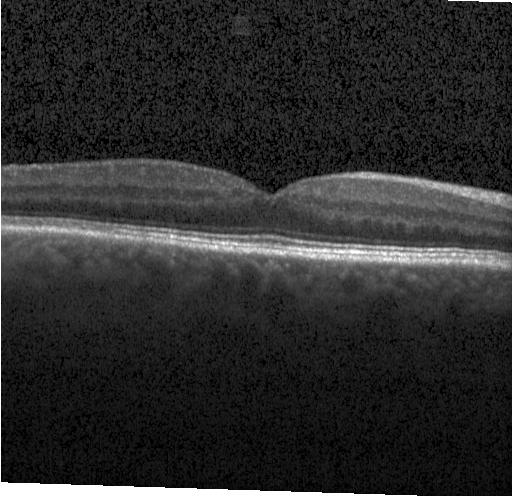
Spectral-domain OCT, optical coherence tomography B-scan, Heidelberg Spectralis. OCT finding: no CNV, DME, or drusen.